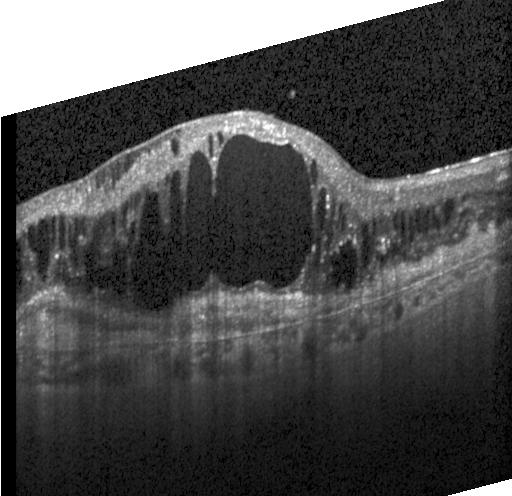
OCT line scan · centered on the fovea · spectral-domain OCT · Heidelberg Spectralis
Finding: choroidal neovascularization (CNV).